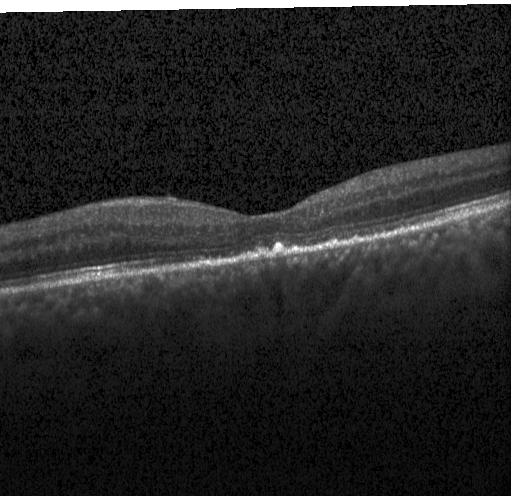
SD-OCT · macular scan · acquired on a Heidelberg Spectralis · retinal OCT cross-section — Impression: multiple drusen.